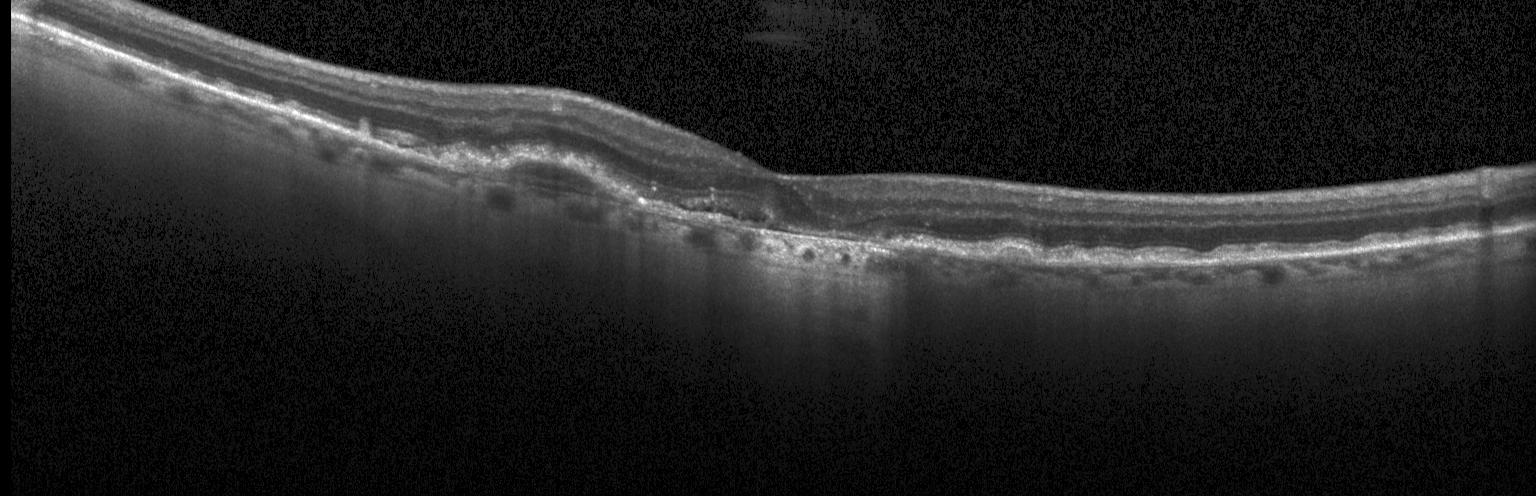 OCT finding: CNV.